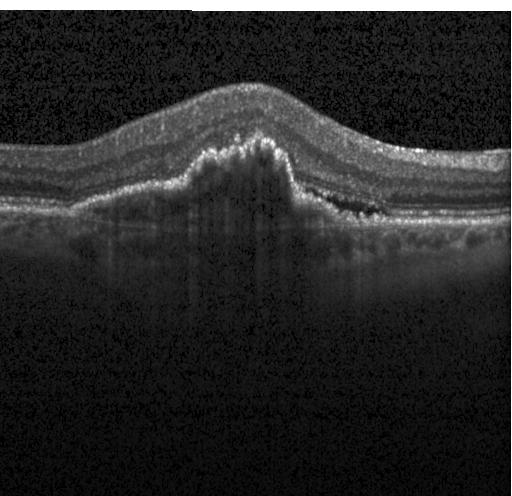 Assessment: choroidal neovascularization (CNV).